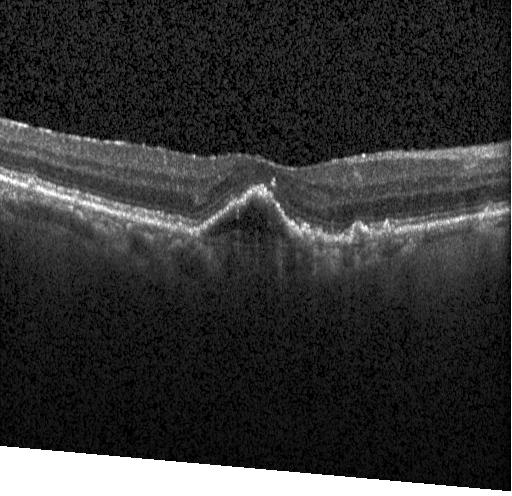 Diagnosis: a choroidal neovascular membrane.